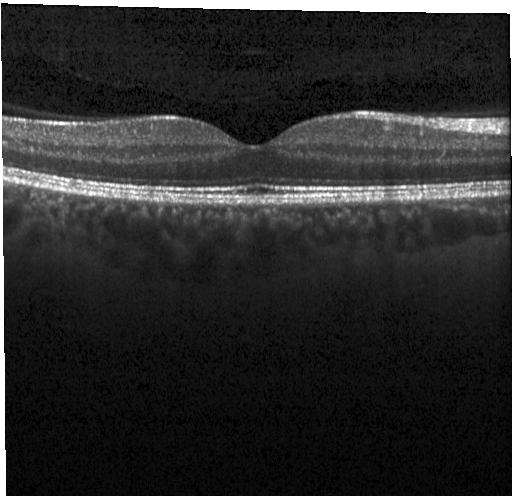
Optical coherence tomography scan · centered on the fovea · acquired on a Heidelberg Spectralis · spectral-domain optical coherence tomography.
Finding: no choroidal neovascularization, diabetic macular edema, or drusen.